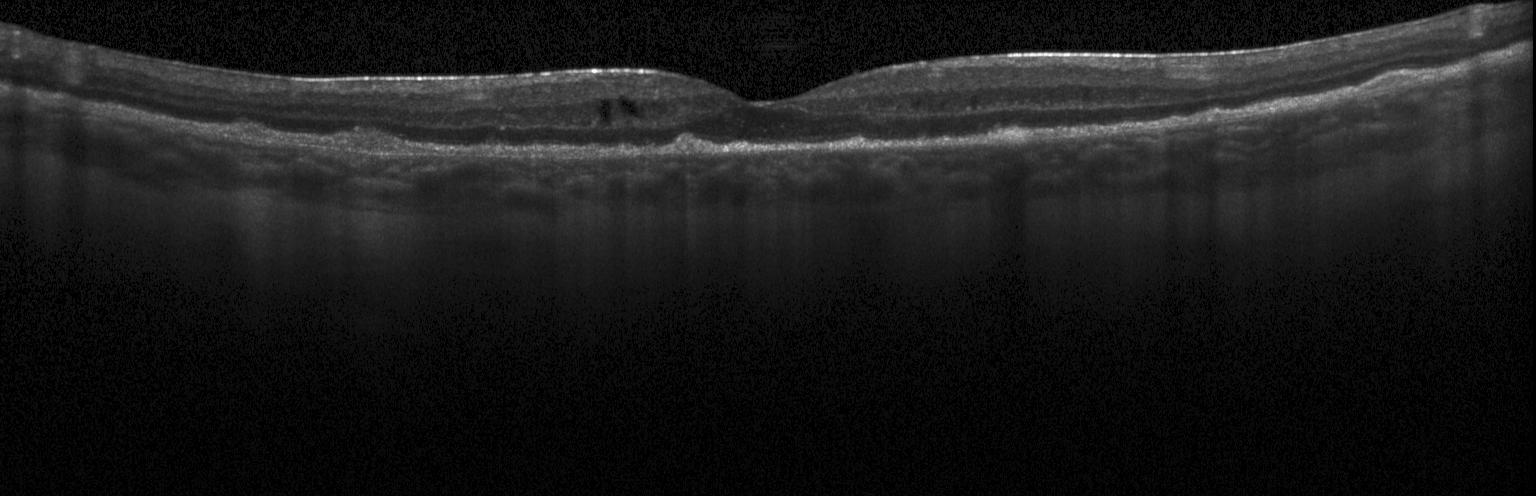
Choroidal neovascularization (CNV).